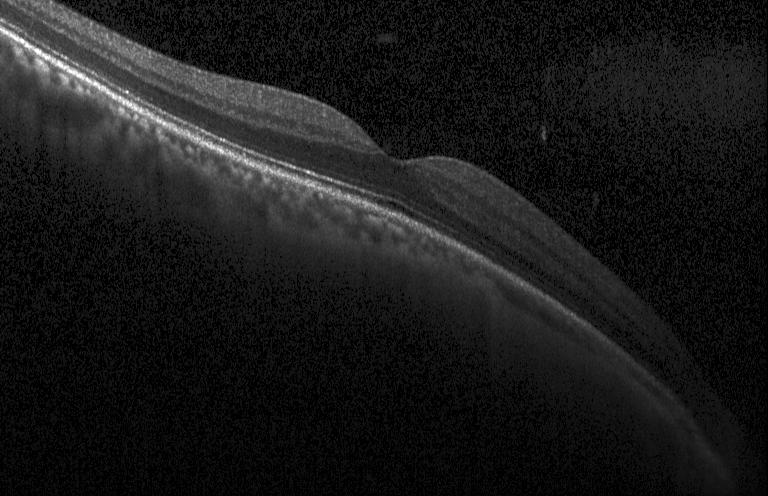 Spectral-domain OCT B-scan: neither choroidal neovascularization, diabetic macular edema, nor drusen.